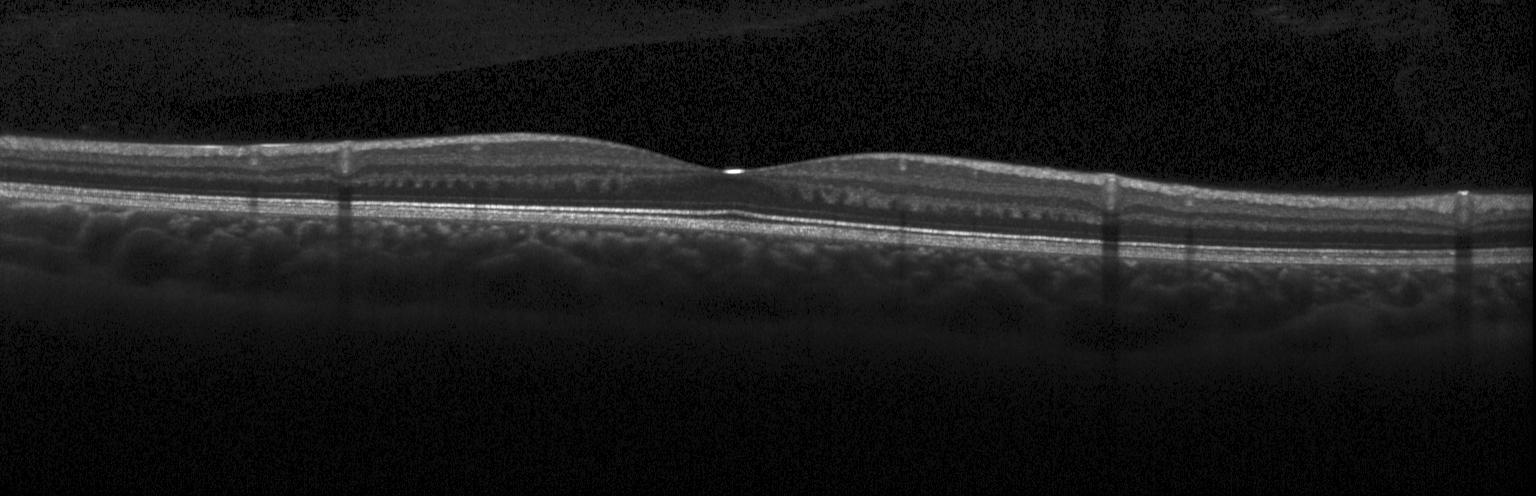 Optical coherence tomography B-scan.
Macular OCT: no choroidal neovascularization, diabetic macular edema, or drusen.